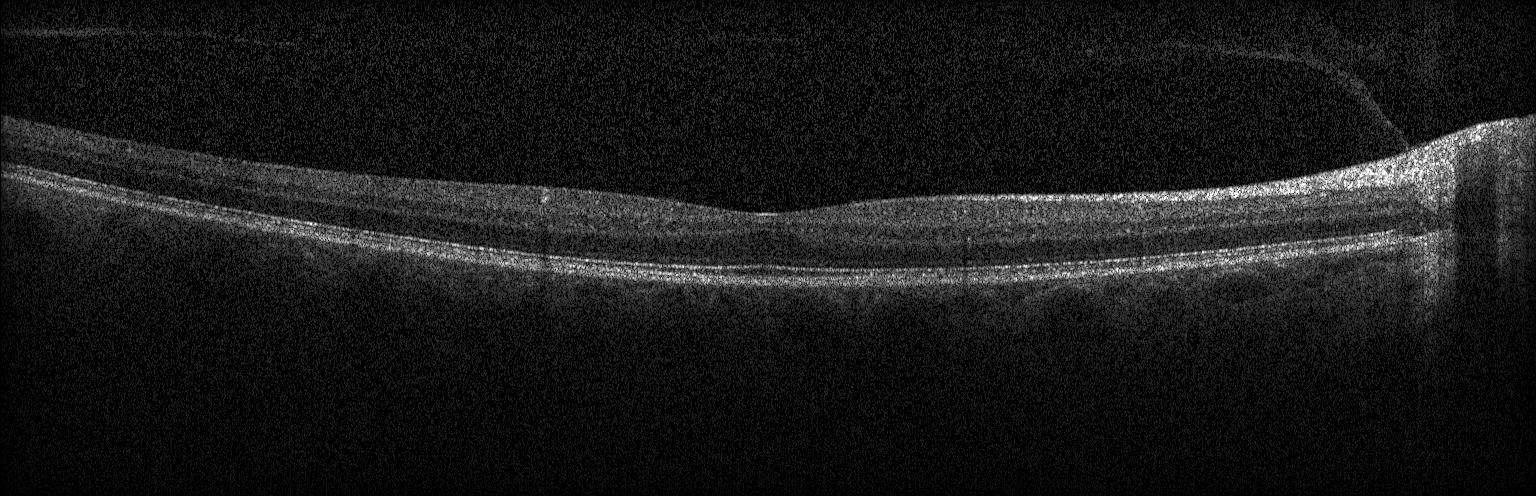
Instrument: Heidelberg Spectralis; retinal OCT cross-section
This B-scan demonstrates no CNV, no DME, and no drusen.